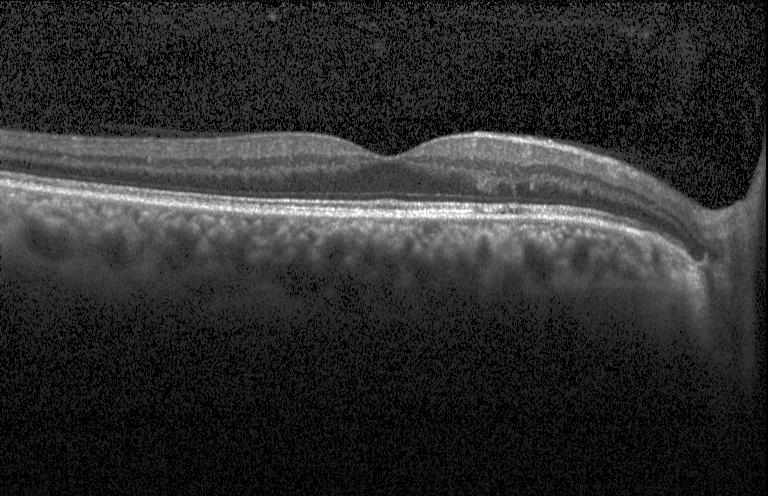
OCT finding: no choroidal neovascularization, no diabetic macular edema, and no drusen.